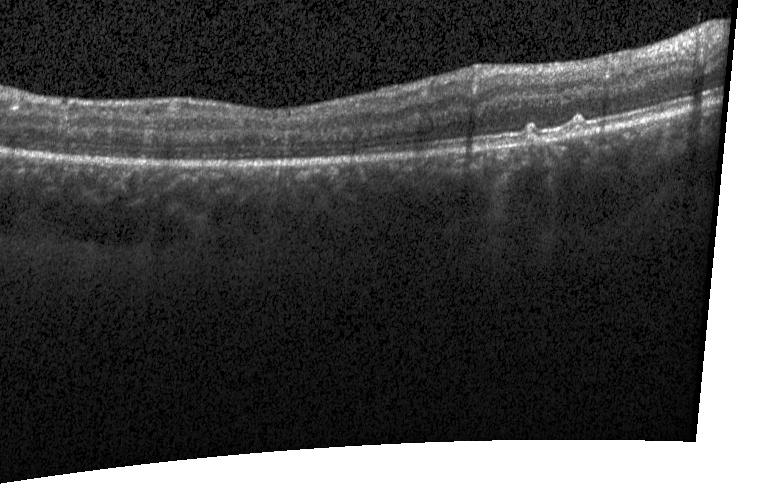 Instrument: Heidelberg Spectralis, SD-OCT, optical coherence tomography B-scan, through the macula.
Macular OCT: drusen.